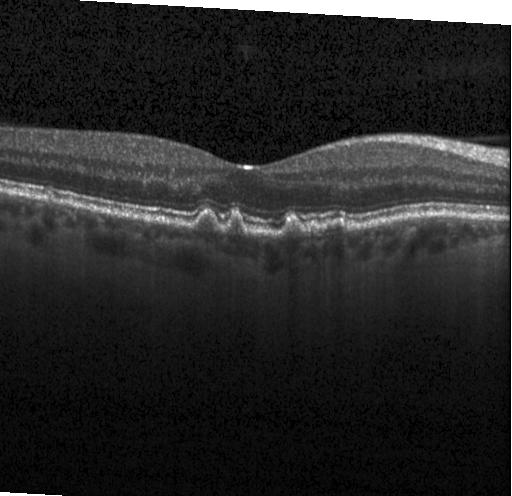

Retinal OCT cross-section · spectral-domain optical coherence tomography · centered on the fovea. Multiple drusen.